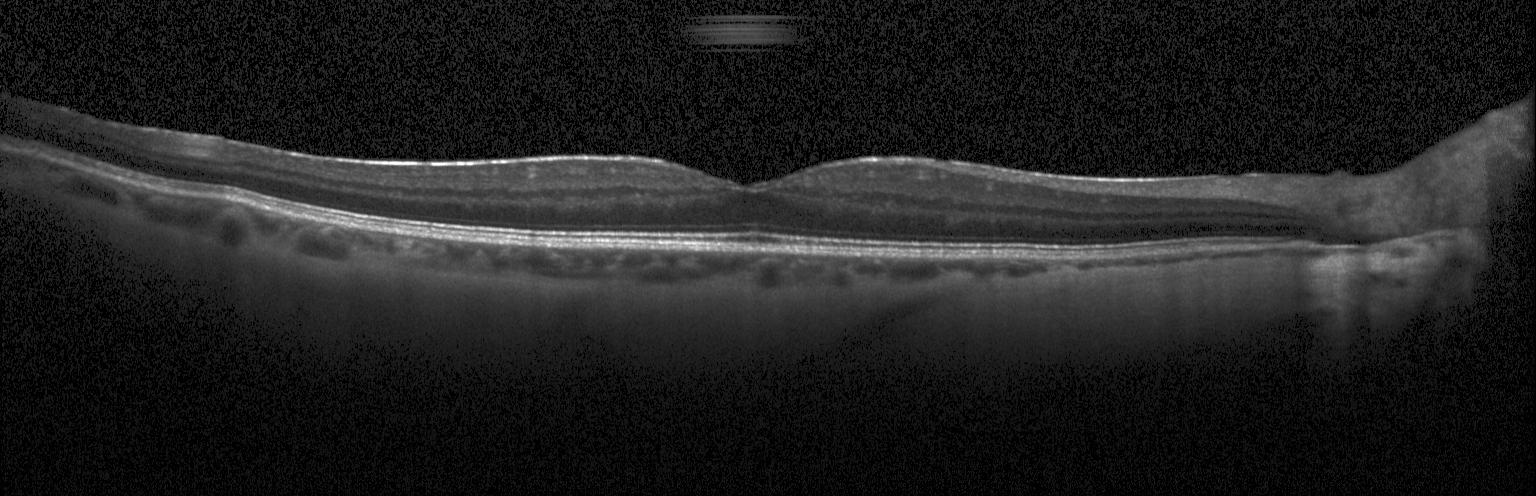 Retinal OCT cross-section
Impression: neither CNV, DME, nor drusen.